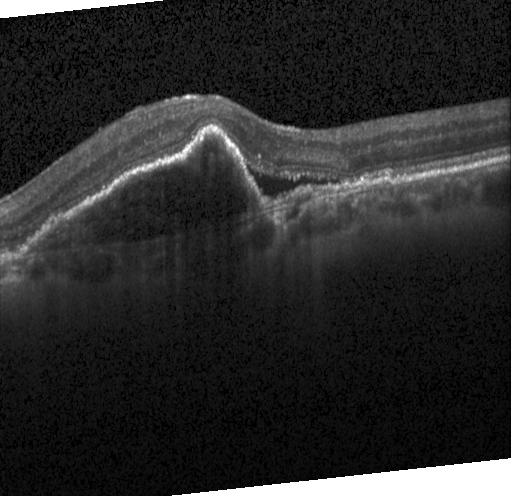

Retinal OCT B-scan
Finding: CNV.